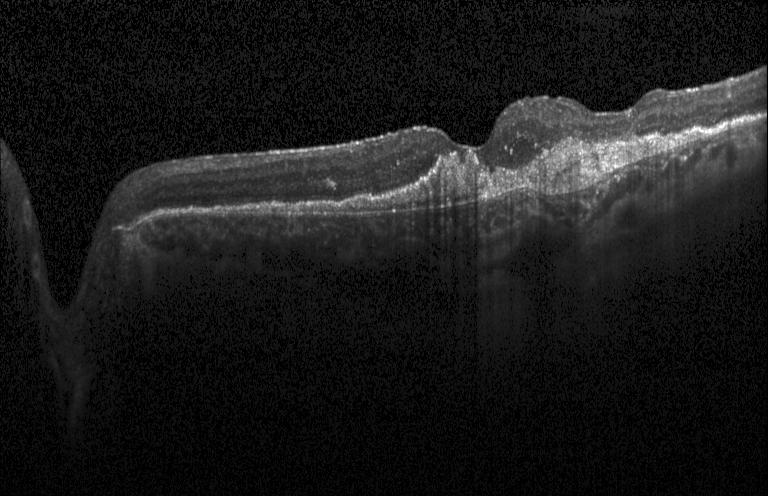
Retinal OCT cross-section
Finding: CNV.